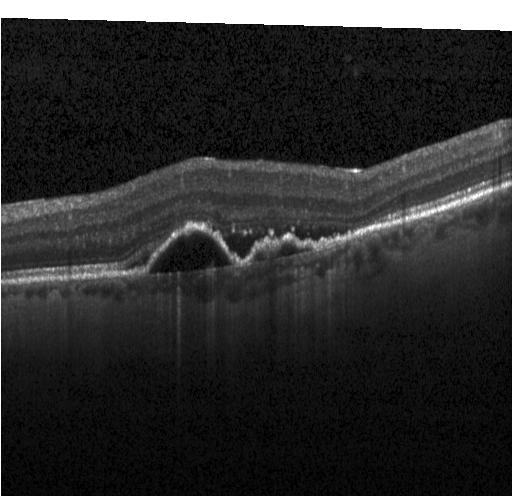 Assessment: CNV.